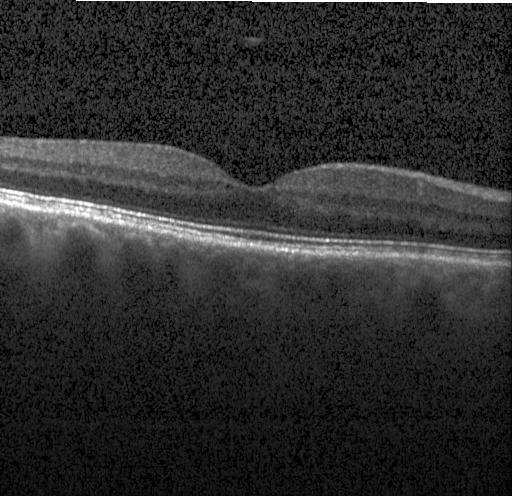 Spectral-domain OCT. Fovea-centered. Optical coherence tomography scan. Acquired on a Heidelberg Spectralis
Neither choroidal neovascularization, diabetic macular edema, nor drusen.